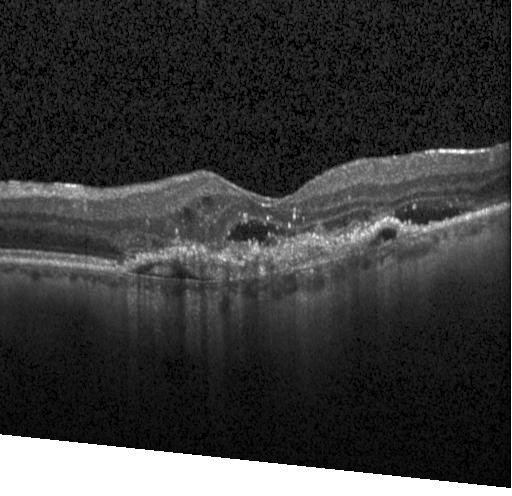

Impression: choroidal neovascularization.